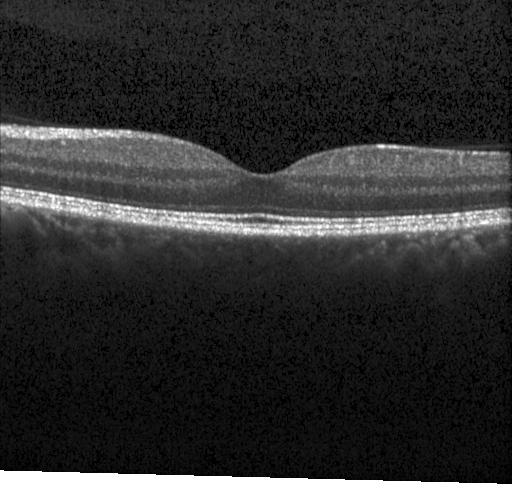 OCT scan showing no choroidal neovascularization, diabetic macular edema, or drusen.